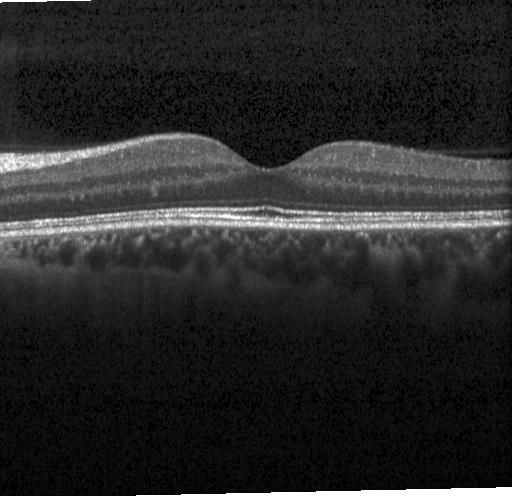

Macular scan, OCT B-scan — No CNV, no DME, and no drusen.